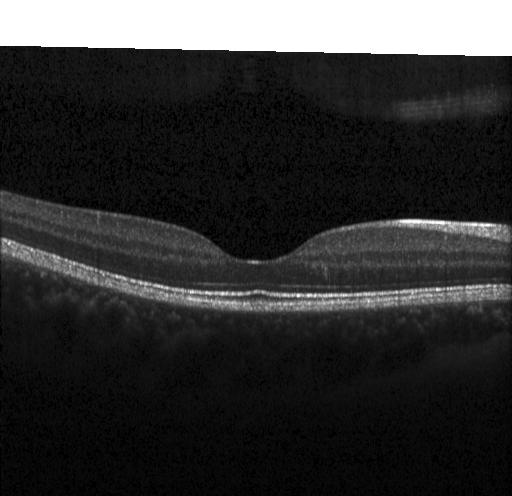
OCT B-scan.
Finding: no choroidal neovascularization, no diabetic macular edema, and no drusen.